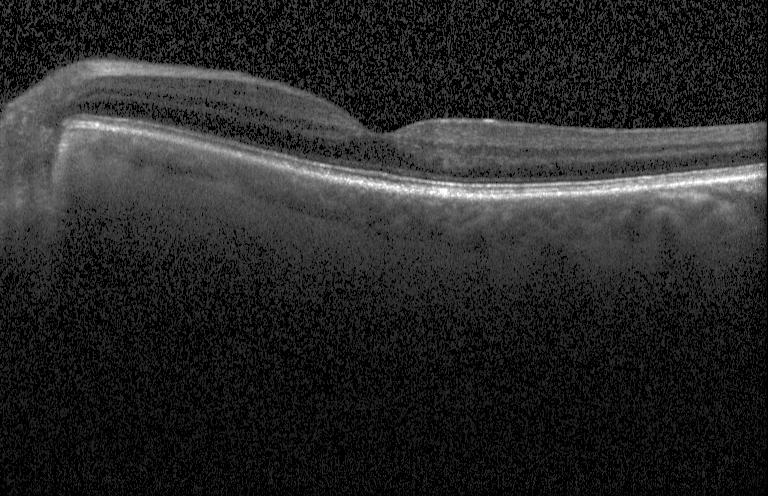
Macular OCT demonstrating no choroidal neovascularization, diabetic macular edema, or drusen.